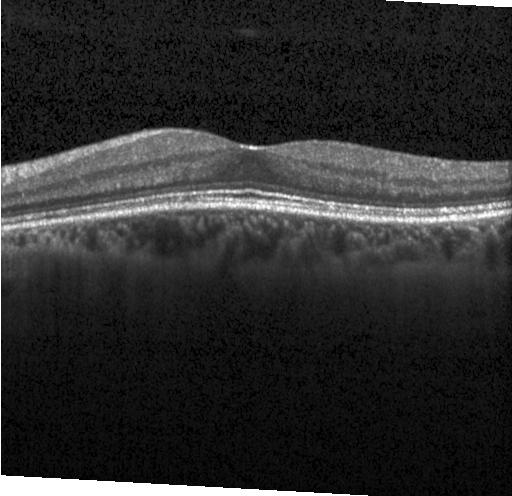

OCT finding: no choroidal neovascularization, no diabetic macular edema, and no drusen.